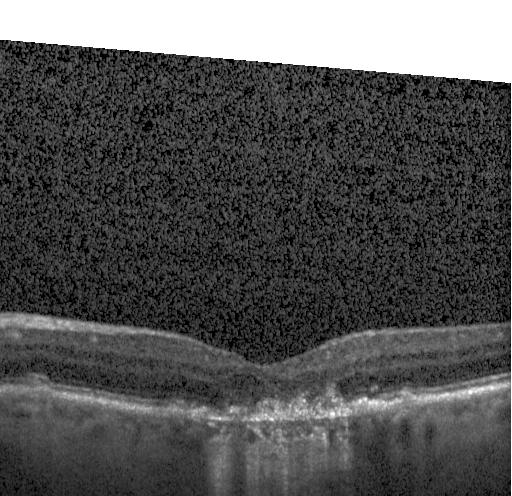
Heidelberg Spectralis OCT system, spectral-domain optical coherence tomography, optical coherence tomography B-scan
This B-scan demonstrates CNV.